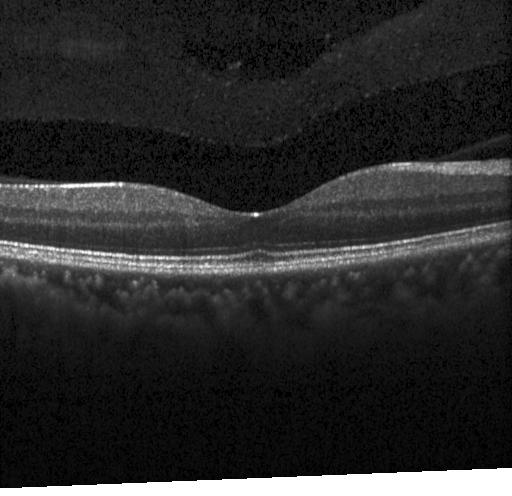

Through the macula, OCT B-scan.
The scan shows no evidence of choroidal neovascularization, diabetic macular edema, or drusen.